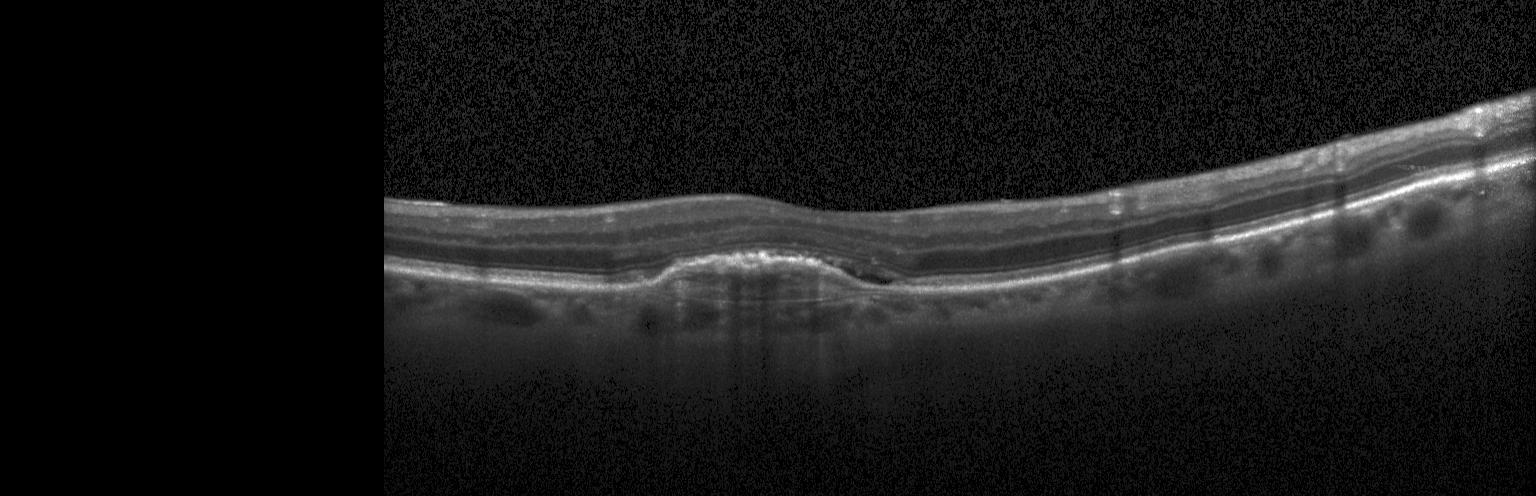
A choroidal neovascular membrane.